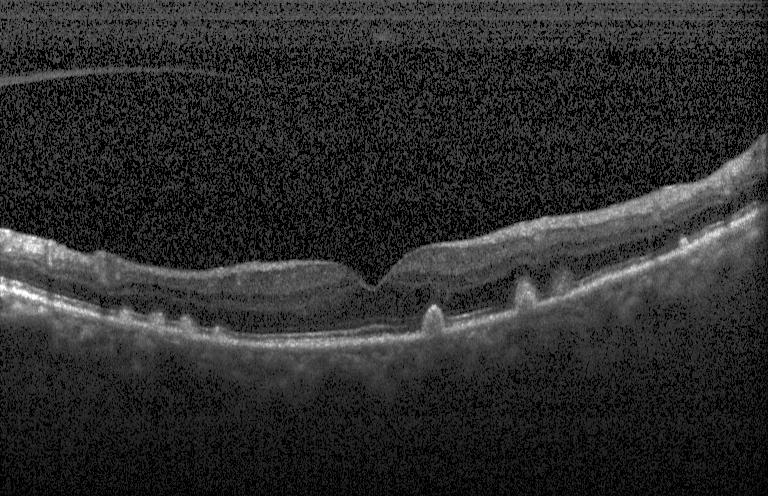

Retinal OCT B-scan.
Dx: multiple drusen.